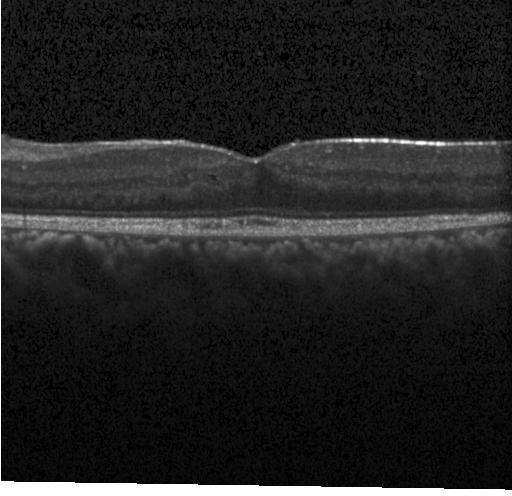
Retinal OCT cross-section showing DME.